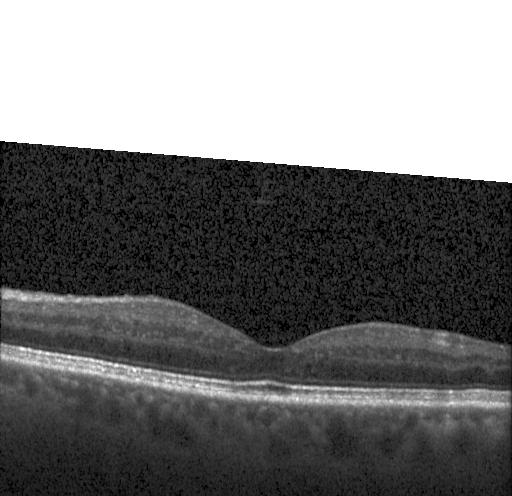
Retinal OCT cross-section; fovea-centered; acquired on a Heidelberg Spectralis. Finding: neither choroidal neovascularization, diabetic macular edema, nor drusen.